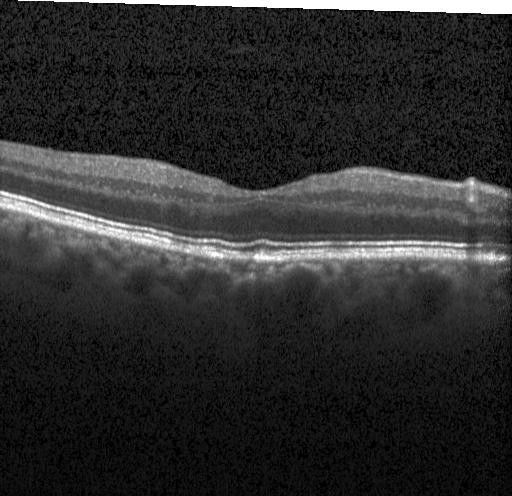 Optical coherence tomography B-scan — Macular OCT: sub-RPE drusenoid deposits.